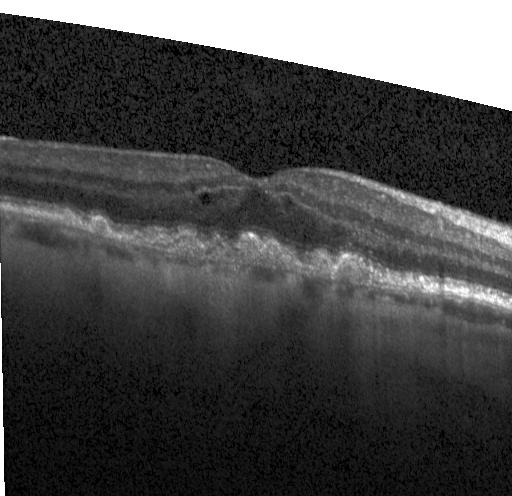 OCT finding: choroidal neovascularization (CNV).